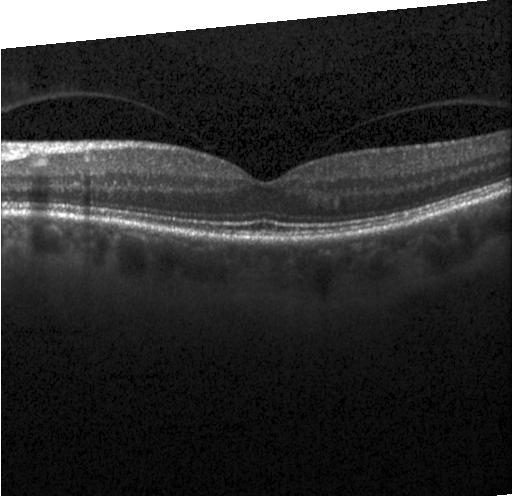
Through the macula, optical coherence tomography scan, spectral-domain OCT — The scan shows neither CNV, DME, nor drusen.